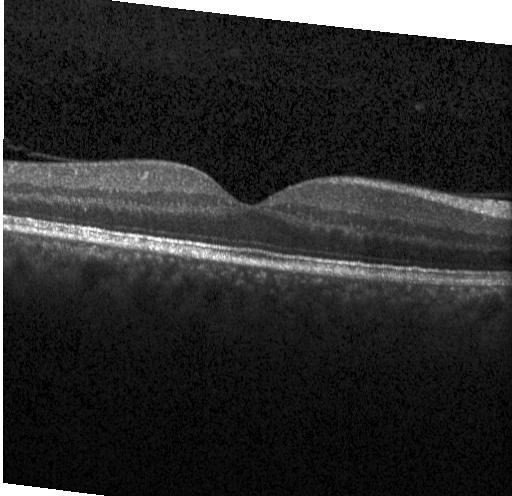
Assessment: no evidence of choroidal neovascularization, diabetic macular edema, or drusen.